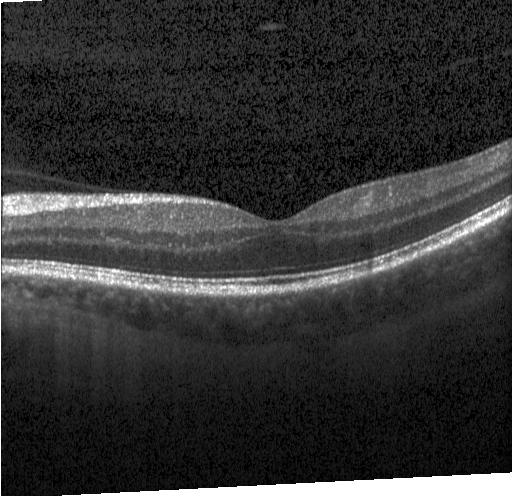
Spectral-domain optical coherence tomography, through the macula, OCT line scan, Heidelberg Spectralis.
No evidence of choroidal neovascularization, diabetic macular edema, or drusen.